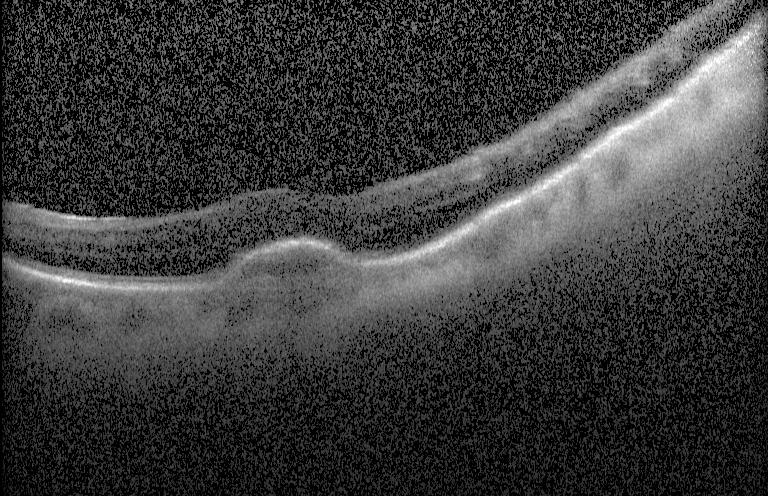 Impression: choroidal neovascularization.